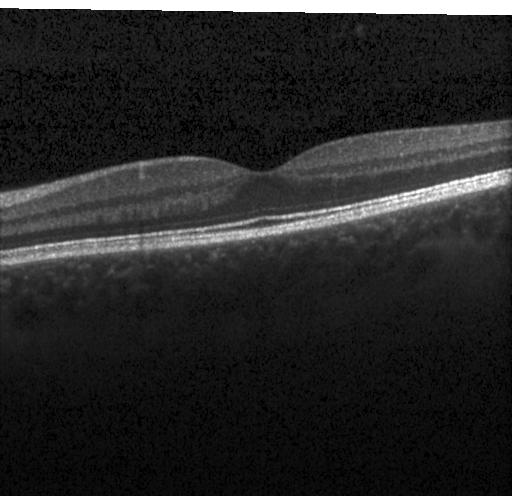
SD-OCT. Retinal OCT B-scan.
OCT finding: neither choroidal neovascularization, diabetic macular edema, nor drusen.